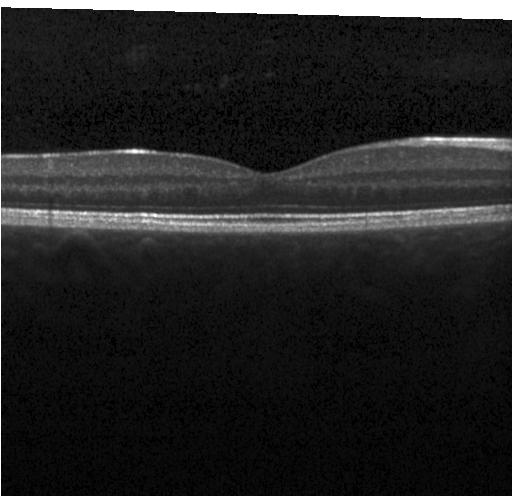
Instrument: Heidelberg Spectralis. OCT B-scan. Dx: no evidence of choroidal neovascularization, diabetic macular edema, or drusen.